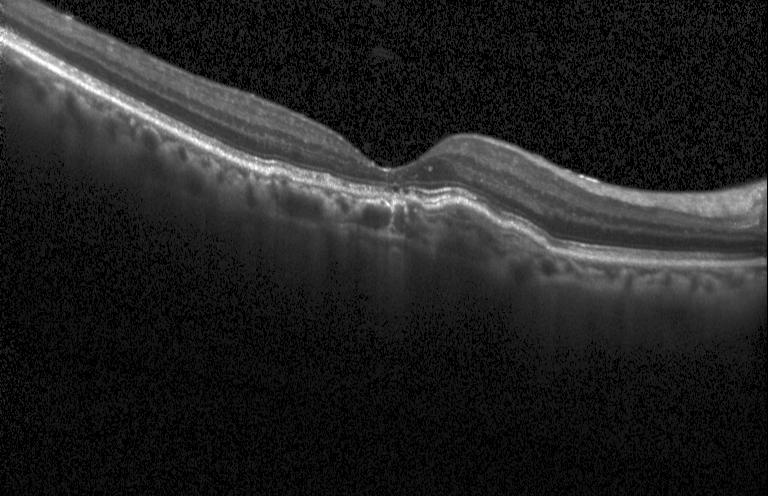 Diagnosis: CNV.